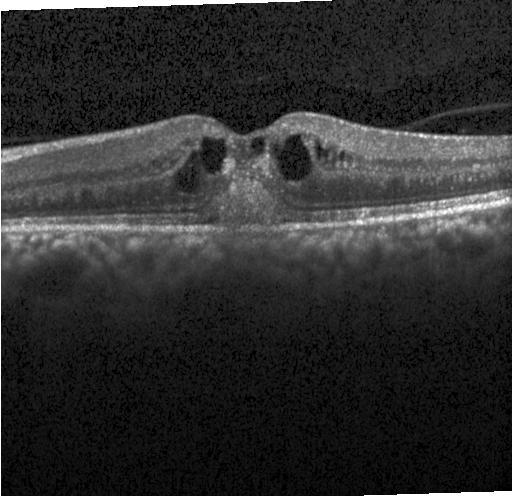

Assessment: a choroidal neovascular membrane.